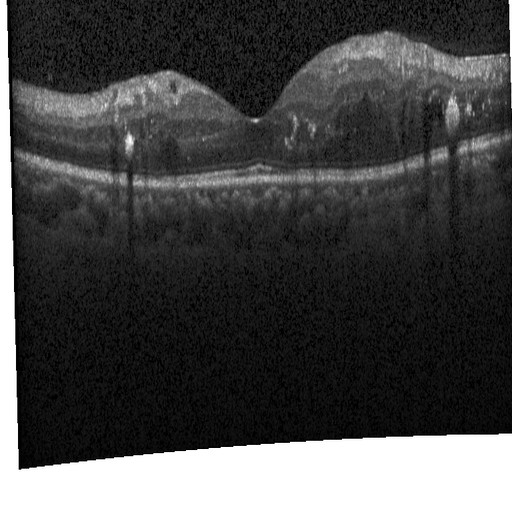
Impression: diabetic macular edema.